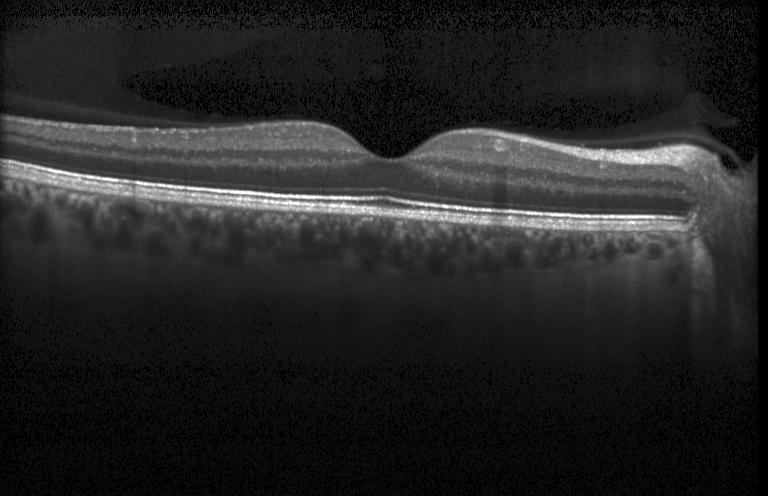
Horizontal scan through the fovea · retinal OCT cross-section · SD-OCT.
Dx: no choroidal neovascularization, diabetic macular edema, or drusen.